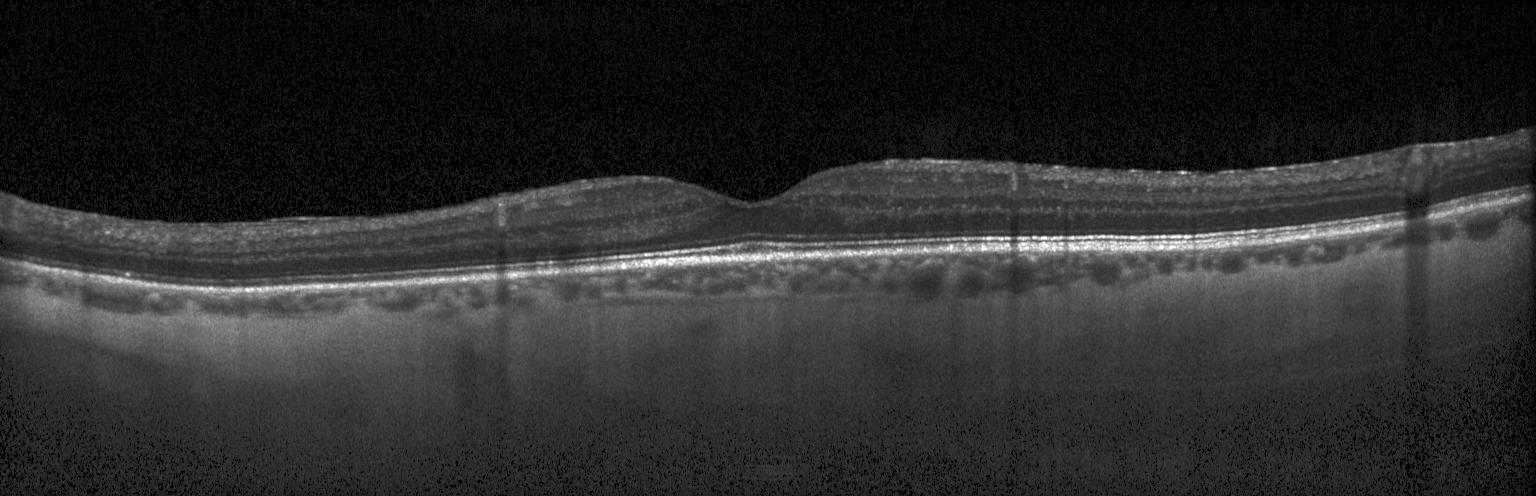
Retinal OCT cross-section. This B-scan demonstrates no choroidal neovascularization, diabetic macular edema, or drusen.